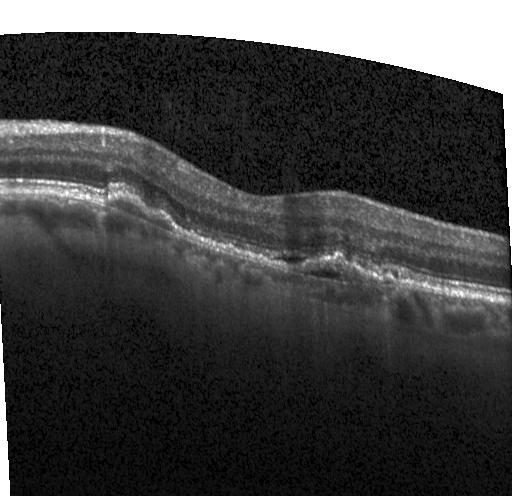 Optical coherence tomography scan; spectral-domain optical coherence tomography.
Impression: a choroidal neovascular membrane.